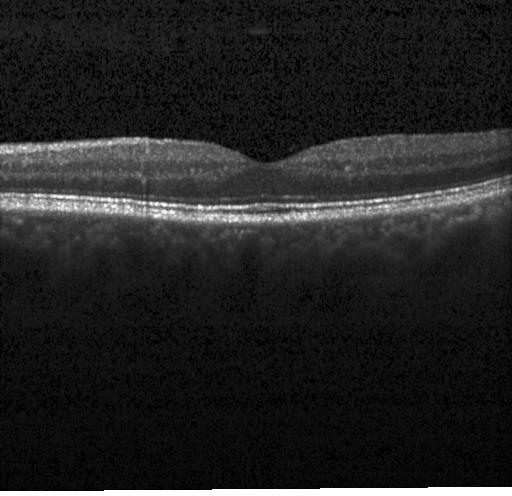
Horizontal scan through the fovea; optical coherence tomography scan.
Diagnosis: neither choroidal neovascularization, diabetic macular edema, nor drusen.